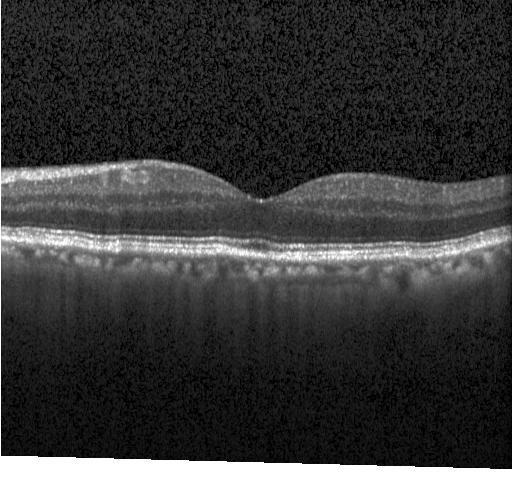
This B-scan demonstrates no choroidal neovascularization, no diabetic macular edema, and no drusen.